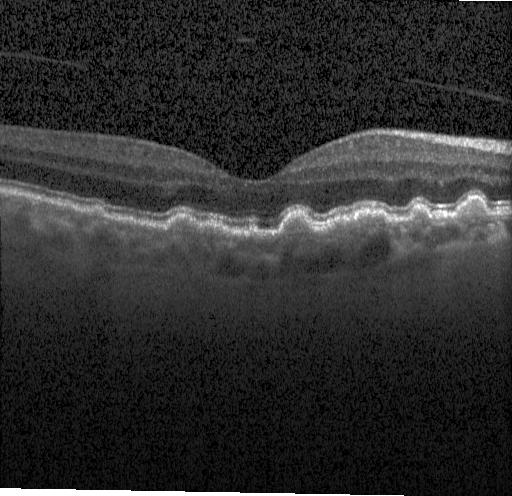

This B-scan demonstrates sub-RPE drusenoid deposits.